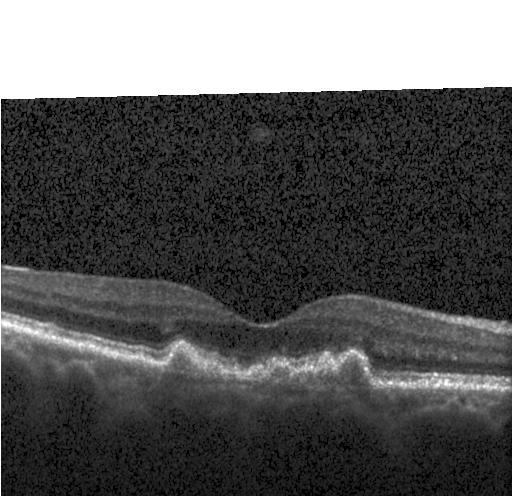 Spectral-domain optical coherence tomography · OCT B-scan
Finding: sub-RPE drusenoid deposits.